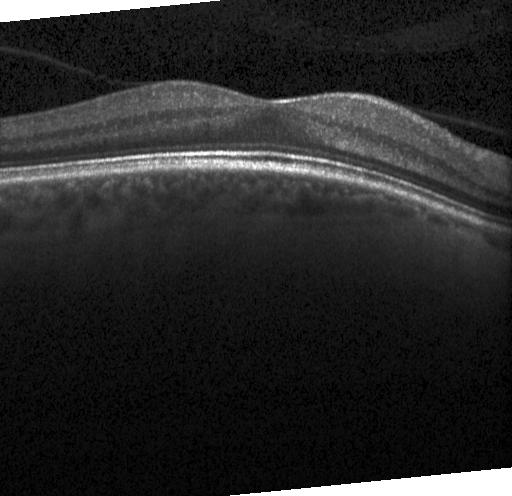 Optical coherence tomography B-scan, acquired on a Heidelberg Spectralis, through the macula. The scan shows no CNV, no DME, and no drusen.